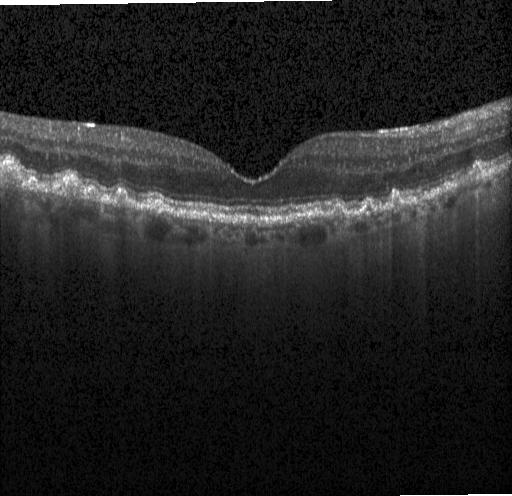 Spectral-domain optical coherence tomography; OCT line scan
Diagnosis: multiple drusen.